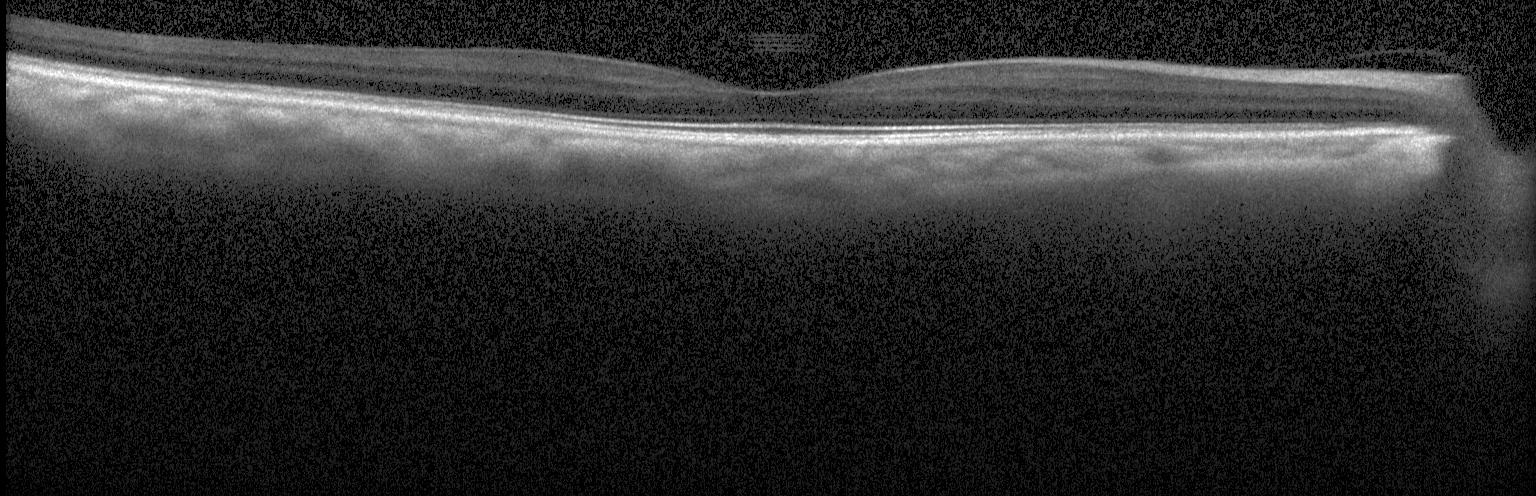

Acquired on a Heidelberg Spectralis; spectral-domain OCT; macular scan; optical coherence tomography scan — Impression: neither choroidal neovascularization, diabetic macular edema, nor drusen.